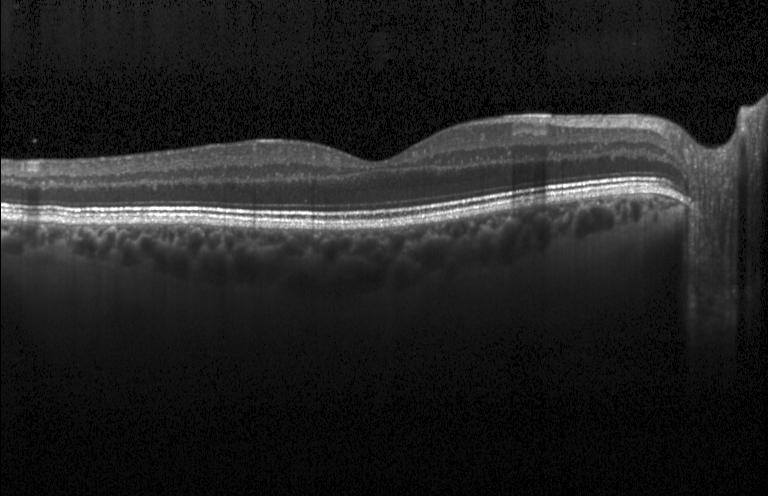
Spectral-domain OCT. Heidelberg Spectralis OCT system. OCT line scan. This B-scan demonstrates no choroidal neovascularization, no diabetic macular edema, and no drusen.